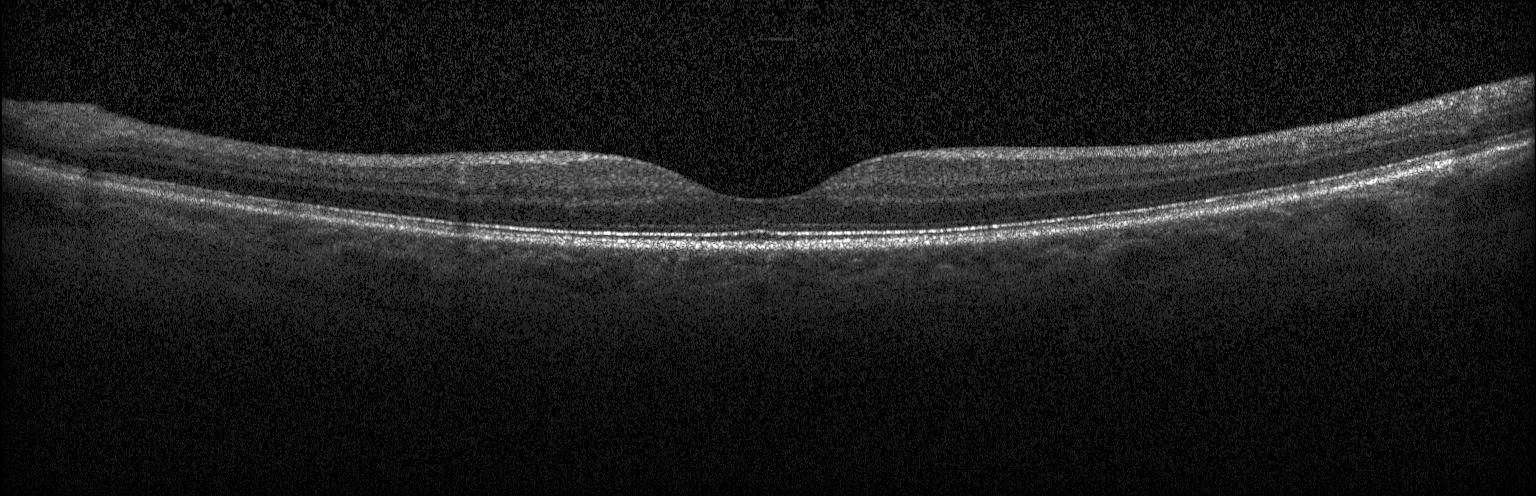

Retinal OCT cross-section. The scan shows no CNV, no DME, and no drusen.